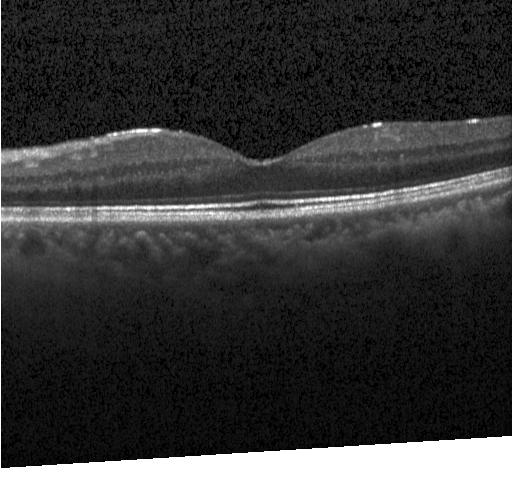

Retinal OCT B-scan, horizontal scan through the fovea, acquired on a Heidelberg Spectralis — The scan shows no CNV, DME, or drusen.